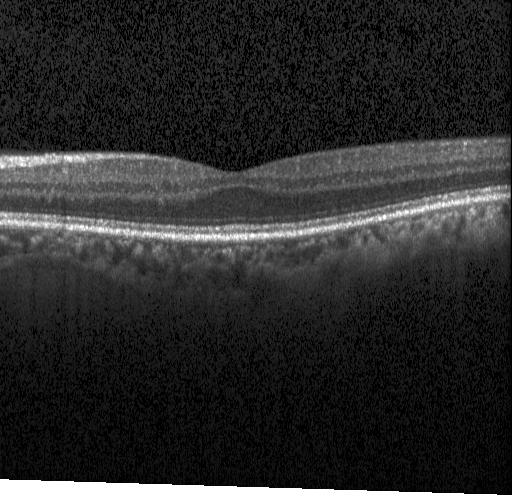

Finding: no evidence of CNV, DME, or drusen.